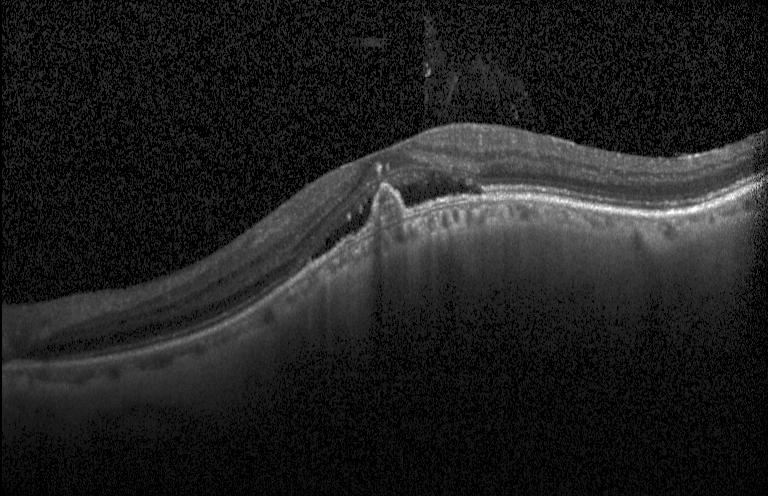

Optical coherence tomography B-scan; fovea-centered; acquired on a Heidelberg Spectralis; spectral-domain OCT
Dx: choroidal neovascularization.